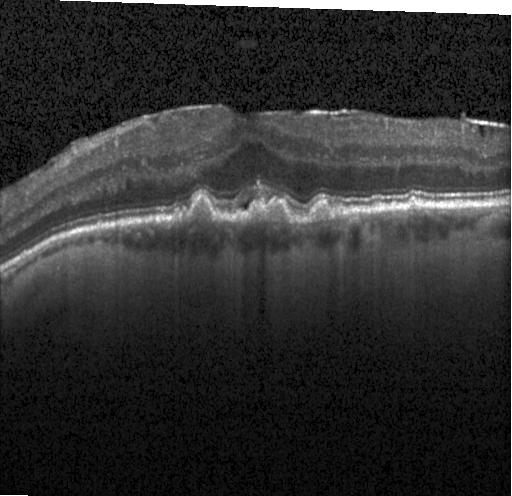
This B-scan demonstrates drusen.